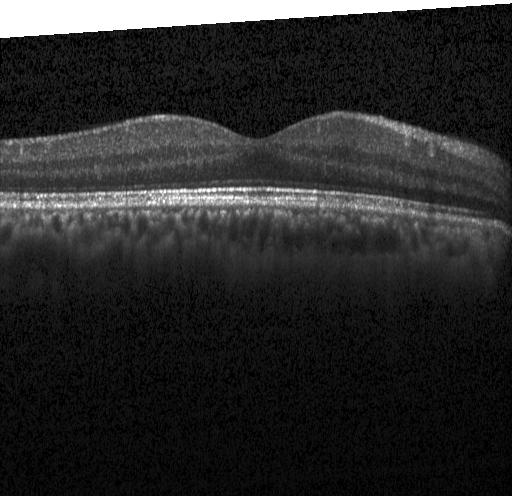
Acquired on a Heidelberg Spectralis. Spectral-domain optical coherence tomography. OCT B-scan.
Diagnosis: no evidence of choroidal neovascularization, diabetic macular edema, or drusen.